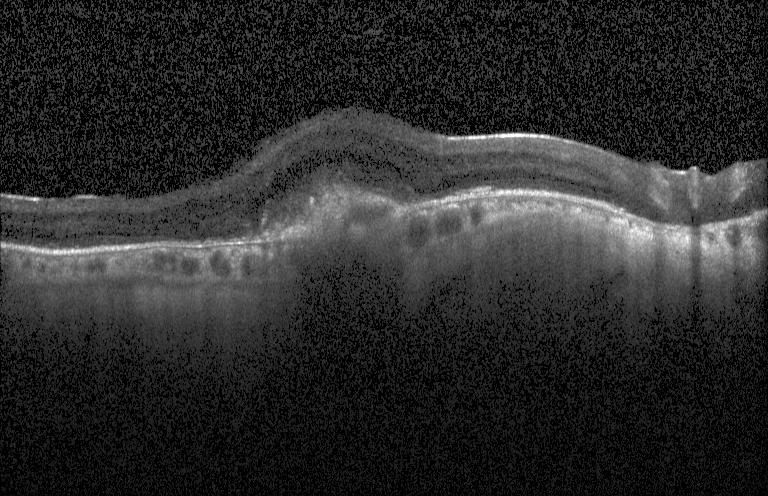
Macular OCT demonstrating a choroidal neovascular membrane.